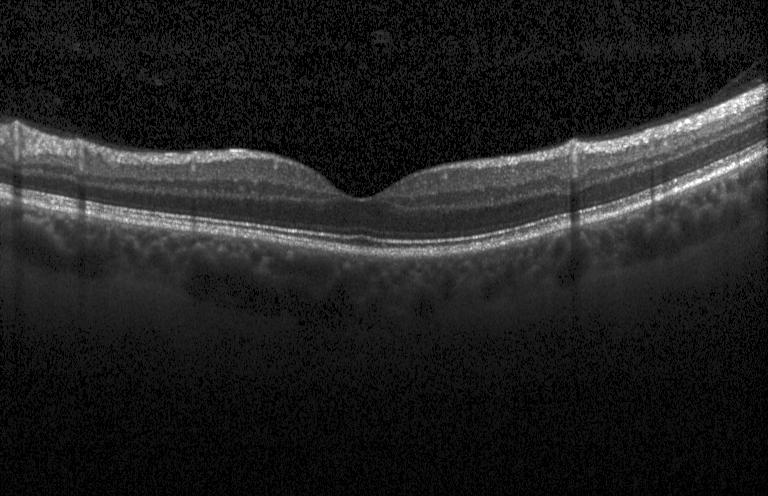 SD-OCT · Heidelberg Spectralis OCT system · retinal OCT cross-section — OCT finding: no evidence of choroidal neovascularization, diabetic macular edema, or drusen.